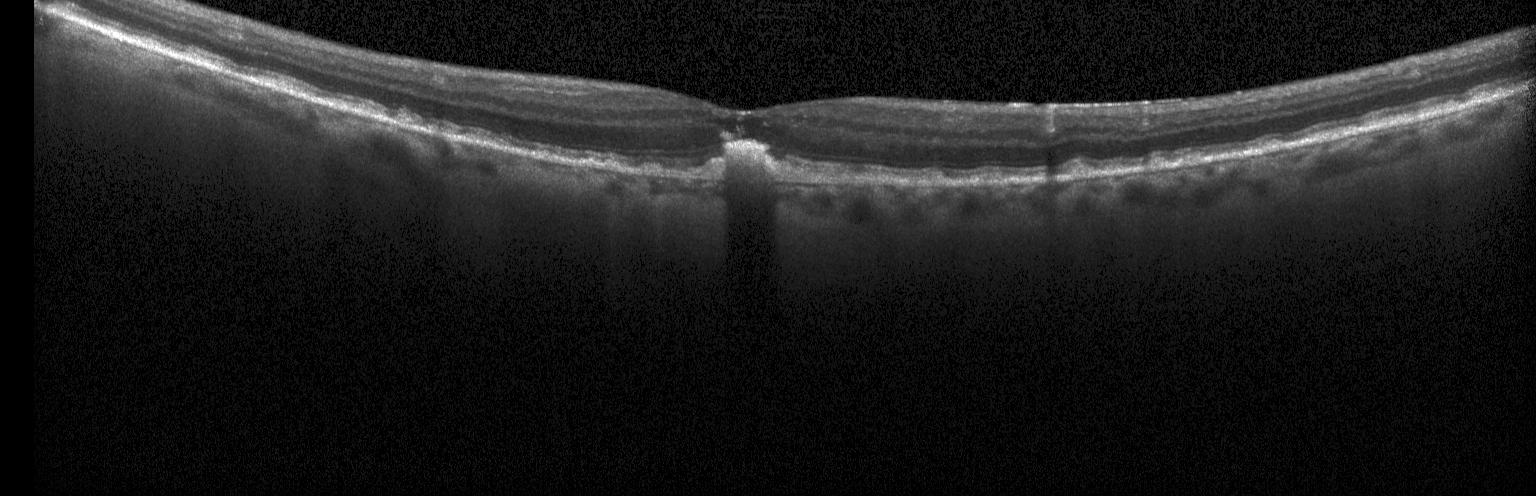
OCT finding: multiple drusen.